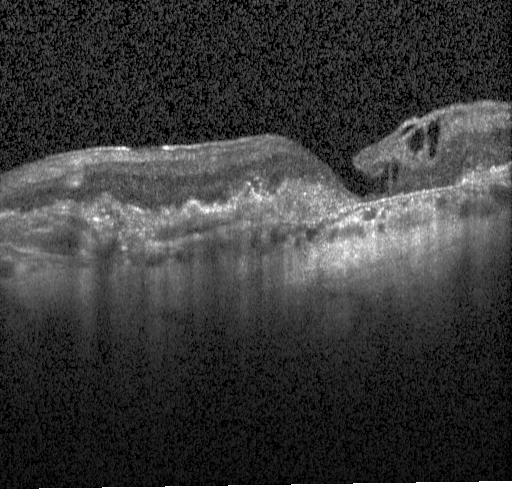 Impression: a choroidal neovascular membrane.